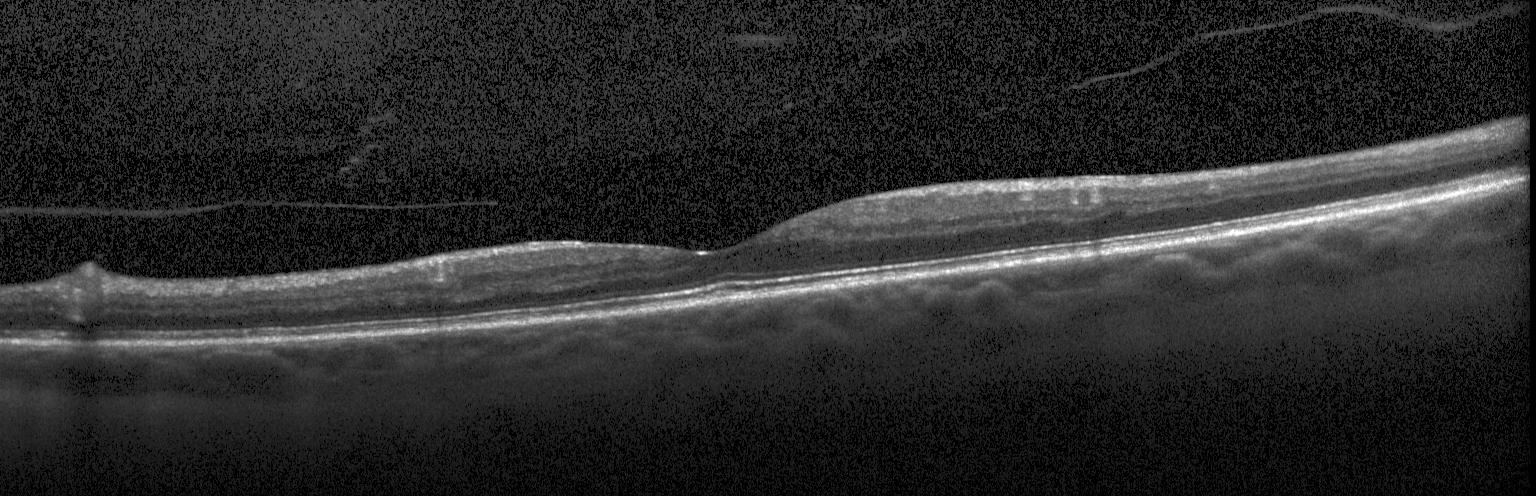
Impression: no evidence of choroidal neovascularization, diabetic macular edema, or drusen.